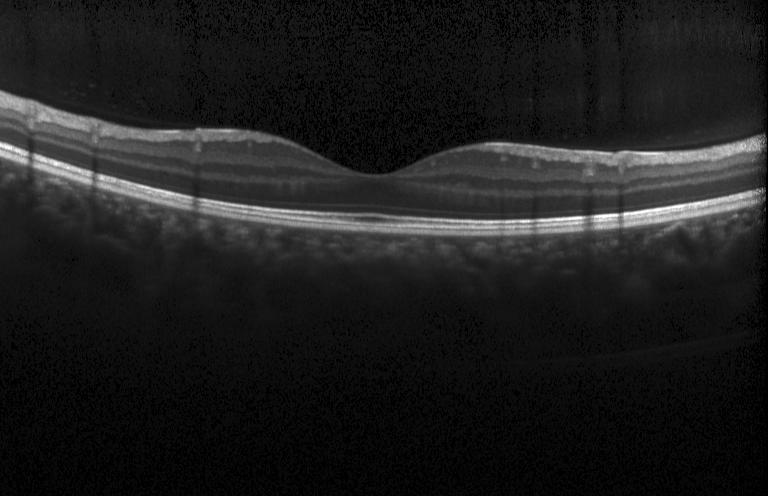
Optical coherence tomography scan. Heidelberg Spectralis OCT system. SD-OCT
OCT finding: no choroidal neovascularization, no diabetic macular edema, and no drusen.